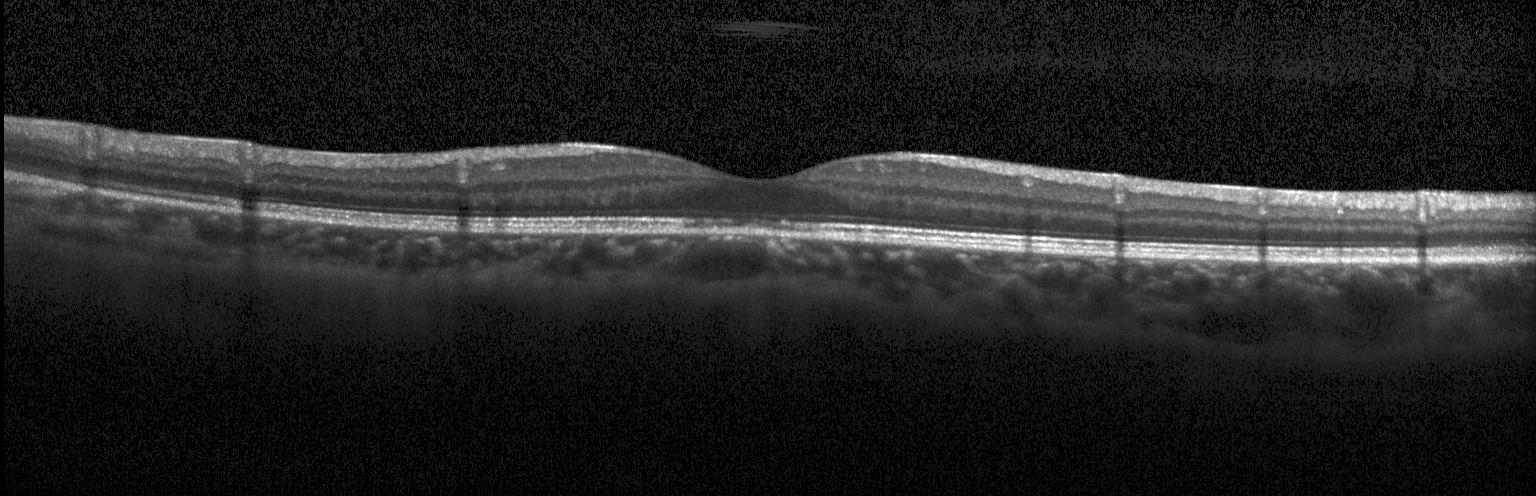
OCT B-scan showing no evidence of CNV, DME, or drusen.